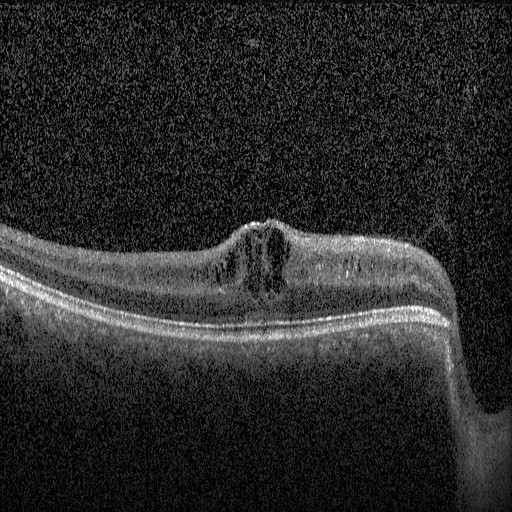
OCT B-scan
Assessment: diabetic macular edema.